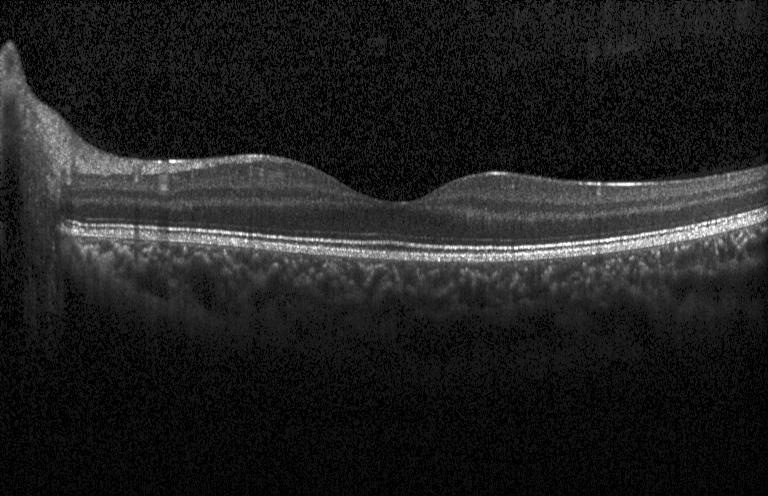
Diagnosis: neither choroidal neovascularization, diabetic macular edema, nor drusen.